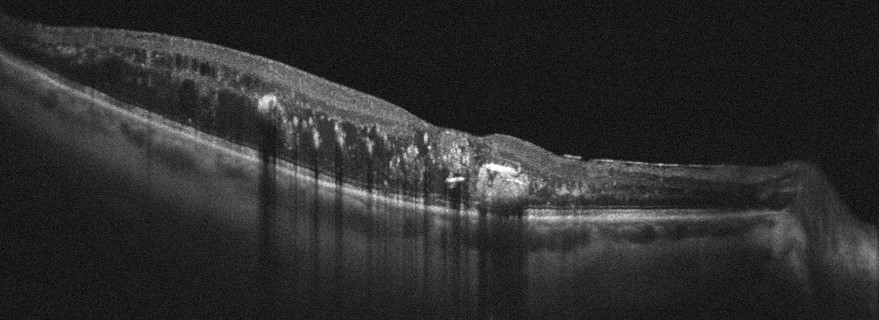
Instrument: Optovue Avanti RTVue XR. Through the macula. Optical coherence tomography B-scan.
Impression: DME.